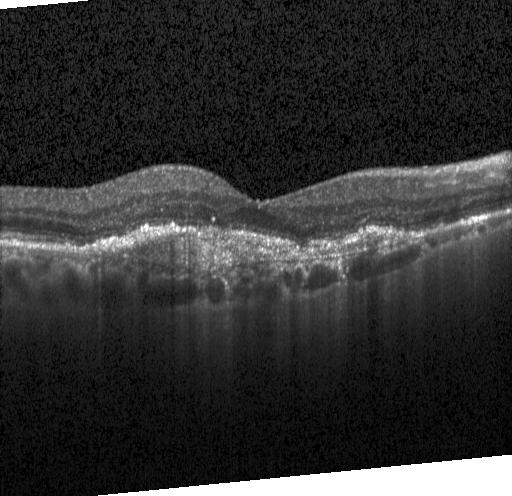
Retinal OCT B-scan · SD-OCT · horizontal scan through the fovea · acquired on a Heidelberg Spectralis. Dx: a choroidal neovascular membrane.